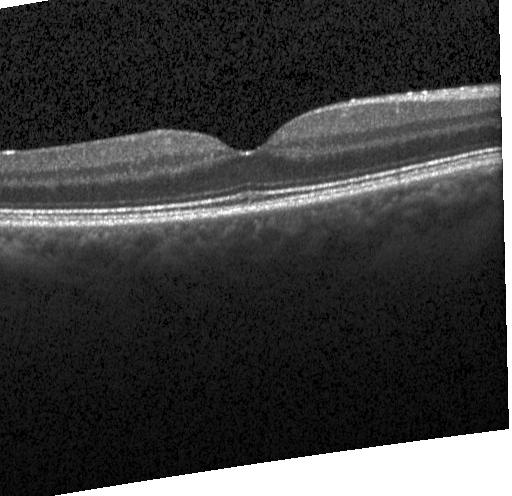
Optical coherence tomography scan, spectral-domain optical coherence tomography.
OCT finding: neither CNV, DME, nor drusen.